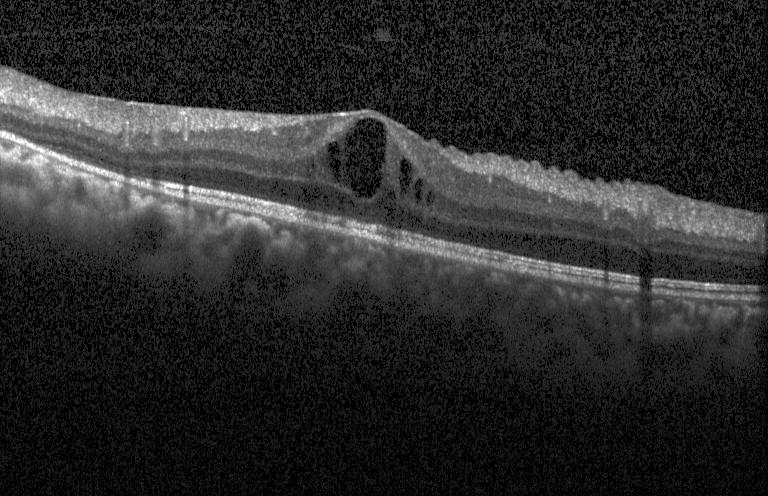 Retinal OCT B-scan. Impression: diabetic macular edema.